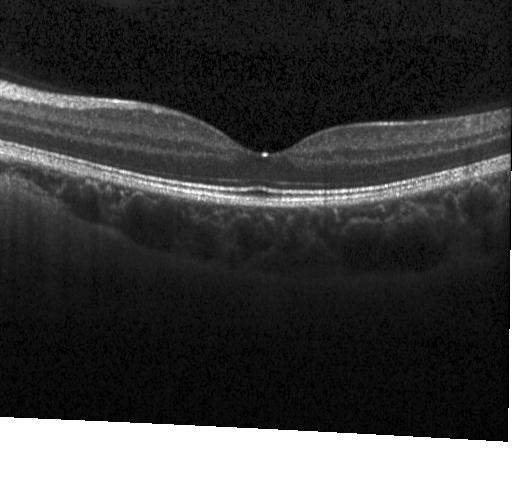 OCT finding: no evidence of choroidal neovascularization, diabetic macular edema, or drusen.